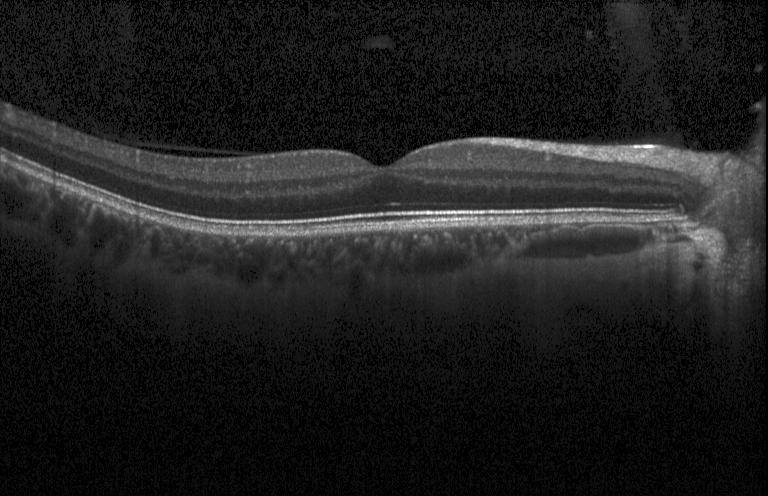

OCT line scan · Heidelberg Spectralis
Impression: no CNV, no DME, and no drusen.